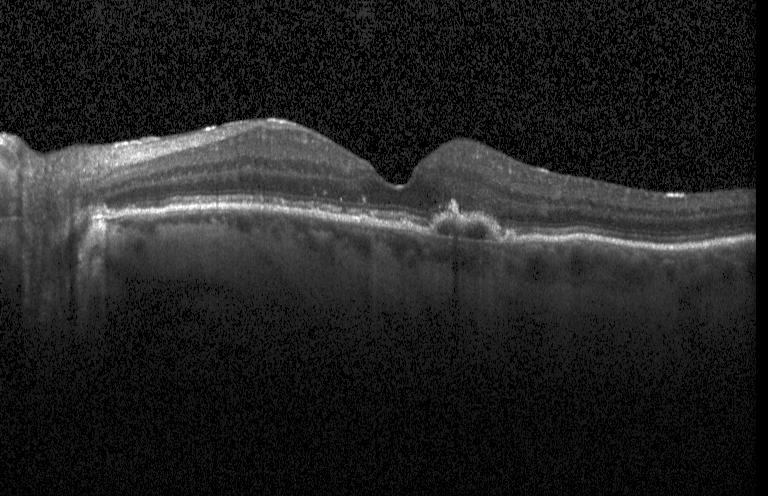
OCT scan showing a choroidal neovascular membrane.